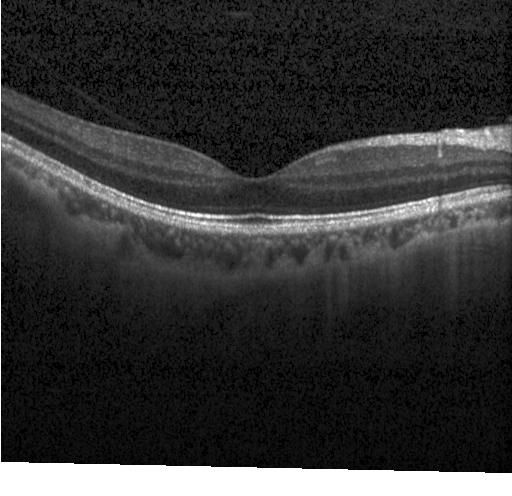 OCT line scan, centered on the fovea, spectral-domain OCT, acquired on a Heidelberg Spectralis
Assessment: no choroidal neovascularization, diabetic macular edema, or drusen.